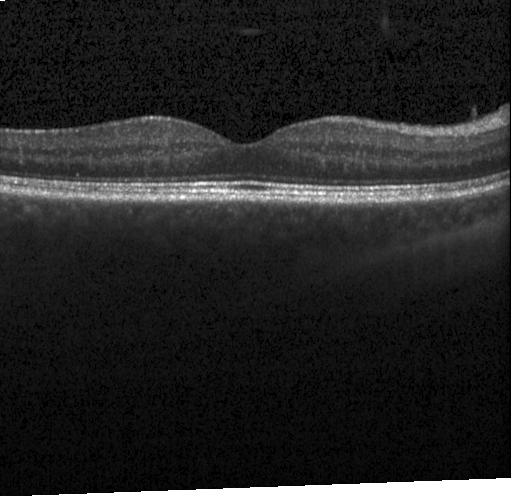

OCT line scan, spectral-domain OCT
Finding: neither CNV, DME, nor drusen.